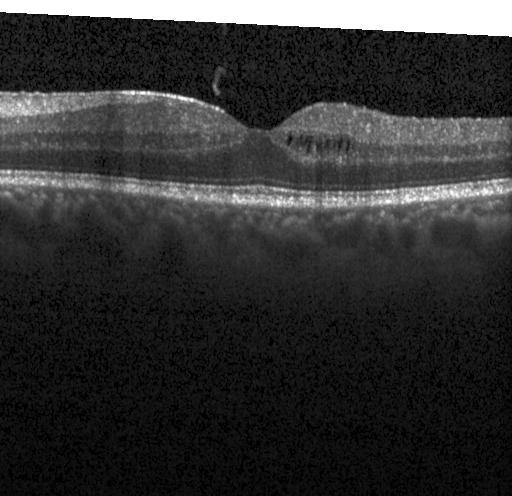 Heidelberg Spectralis OCT system. Spectral-domain optical coherence tomography. Retinal OCT cross-section.
Dx: DME.